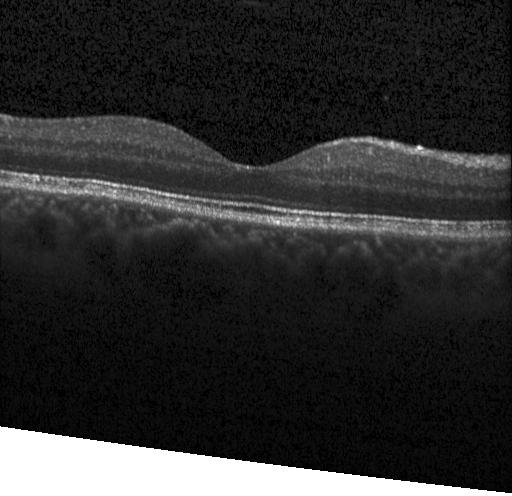 Finding: no evidence of choroidal neovascularization, diabetic macular edema, or drusen.